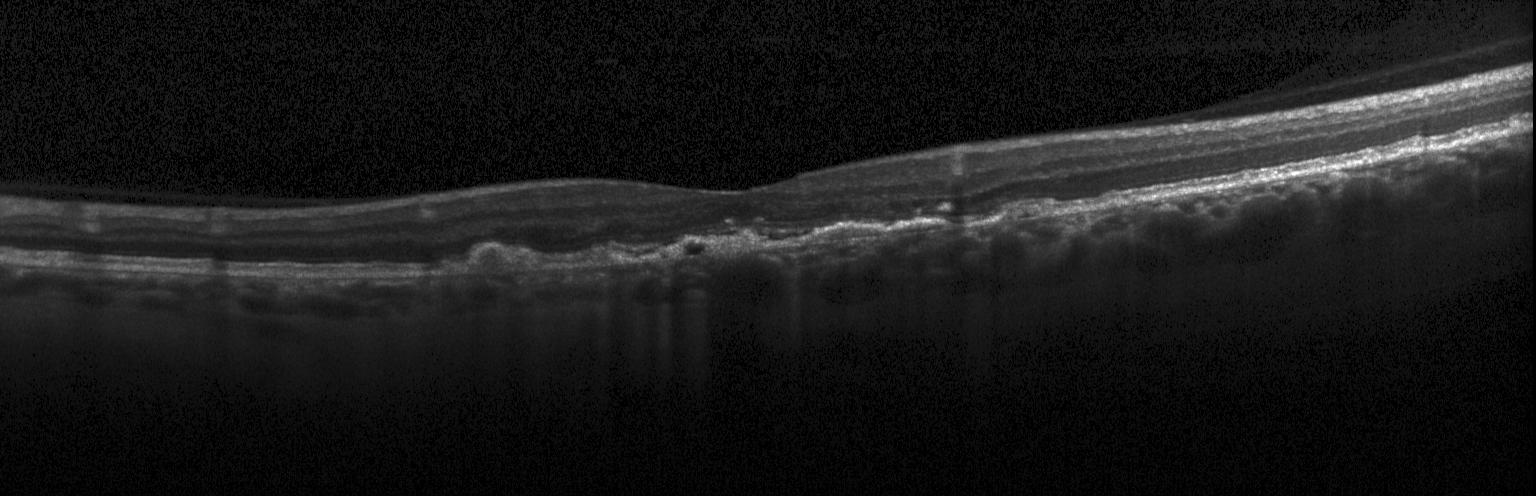

Spectral-domain optical coherence tomography; instrument: Heidelberg Spectralis; optical coherence tomography scan.
Dx: a choroidal neovascular membrane.